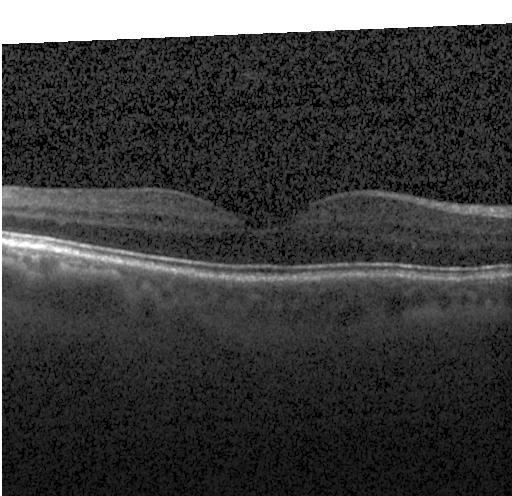 Dx: no CNV, DME, or drusen.